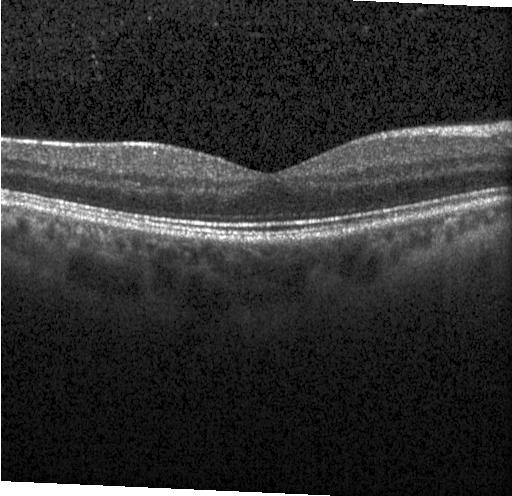 No evidence of choroidal neovascularization, diabetic macular edema, or drusen.